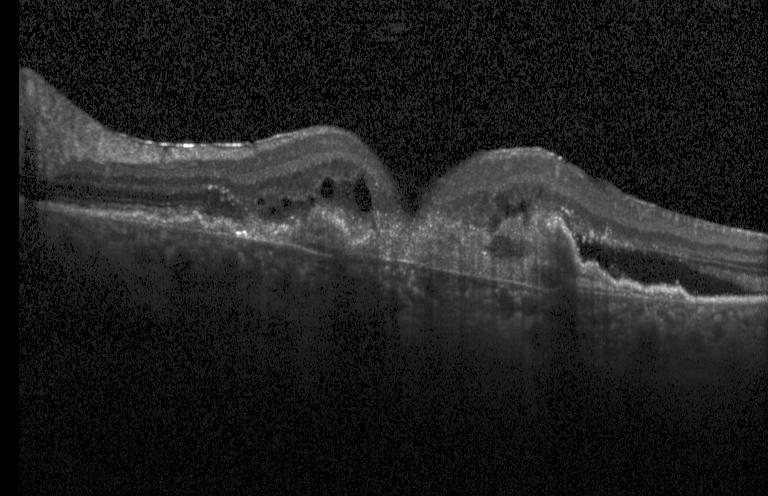 This B-scan demonstrates a choroidal neovascular membrane.